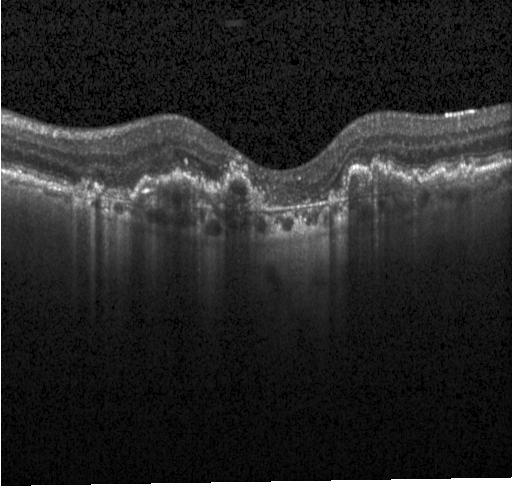 Spectral-domain OCT · optical coherence tomography B-scan · instrument: Heidelberg Spectralis
Assessment: choroidal neovascularization (CNV).